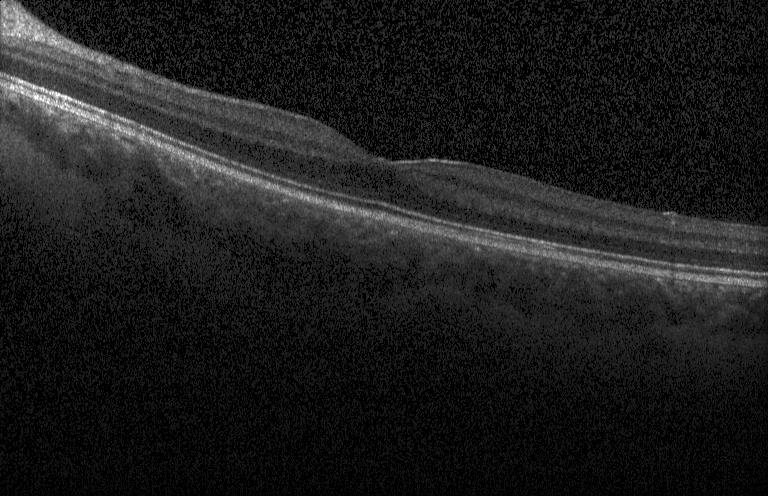

Macular OCT demonstrating no choroidal neovascularization, diabetic macular edema, or drusen.